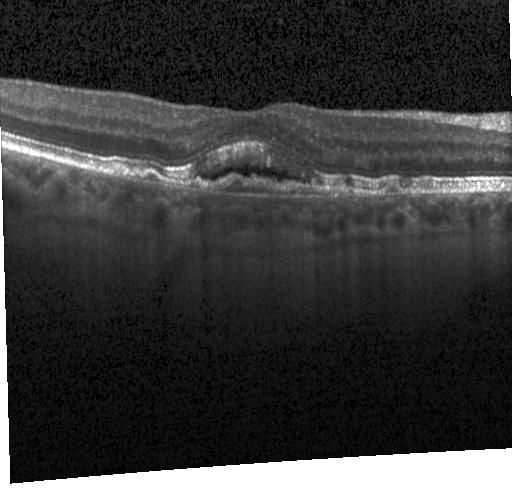

Finding: choroidal neovascularization.